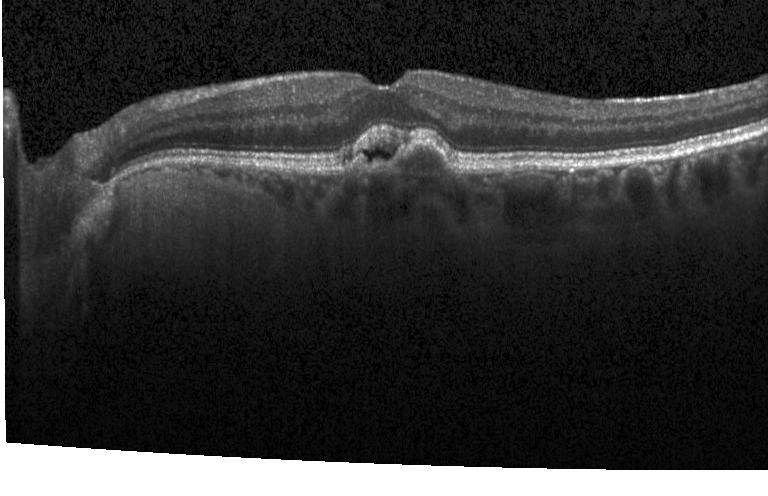

OCT B-scan showing a choroidal neovascular membrane.